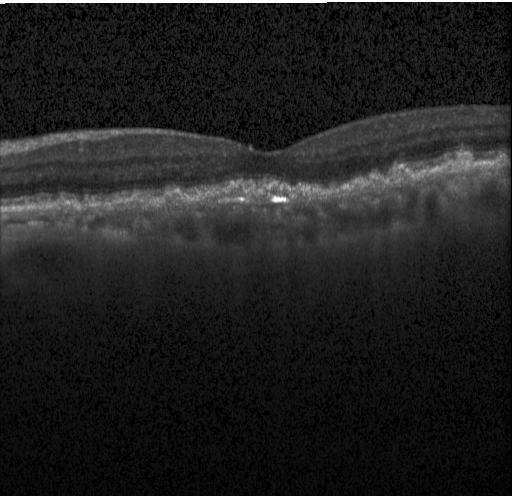

Heidelberg Spectralis OCT system, spectral-domain OCT, OCT B-scan.
Impression: multiple drusen.